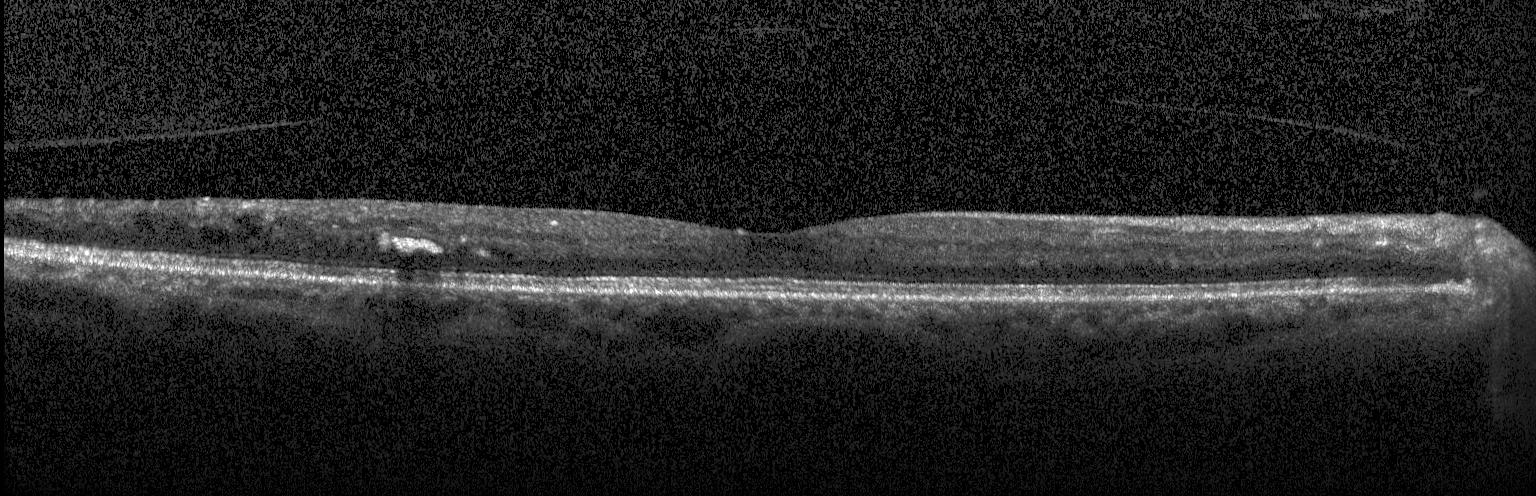 Diagnosis: diabetic macular edema (DME).